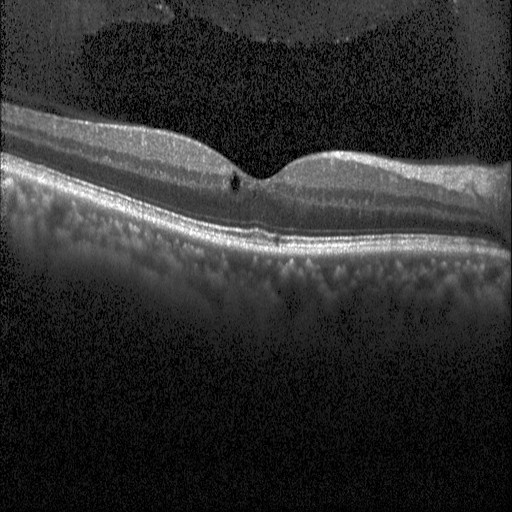 Macular scan; spectral-domain optical coherence tomography; retinal OCT cross-section; Heidelberg Spectralis OCT system. Impression: diabetic macular edema.